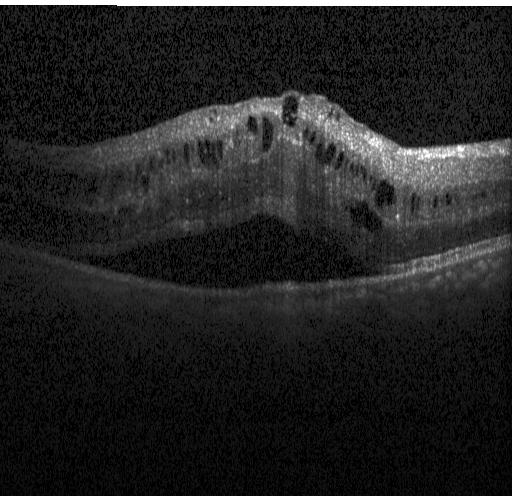

Diabetic macular edema (DME).